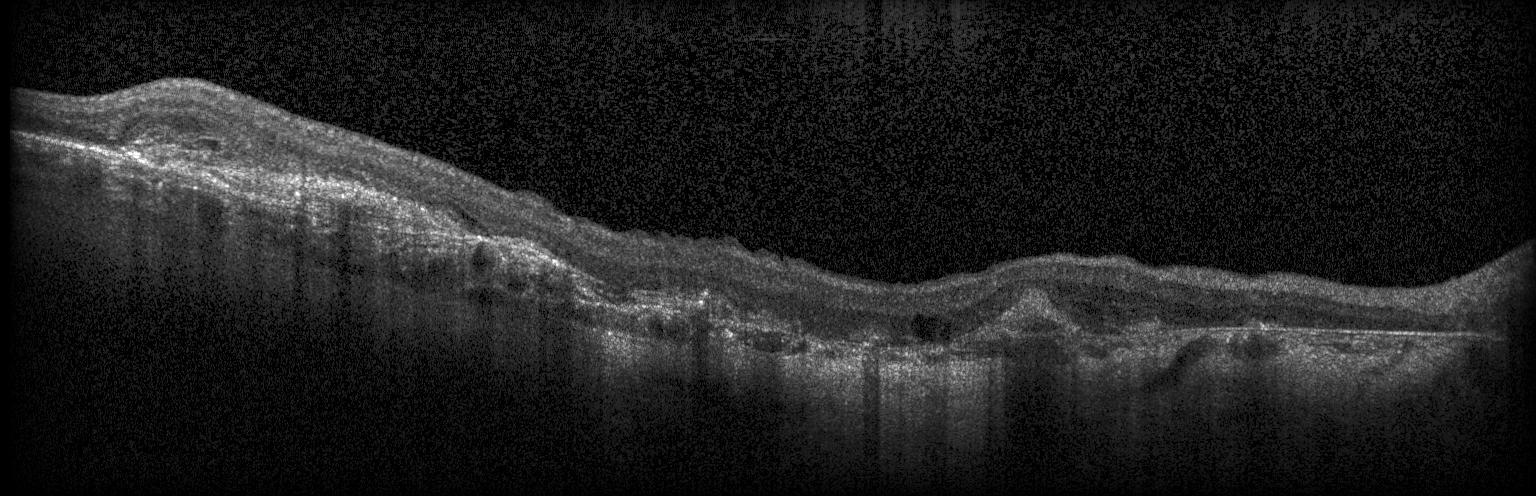
Heidelberg Spectralis OCT system. Retinal OCT cross-section. Through the macula. Spectral-domain OCT — Impression: choroidal neovascularization (CNV).